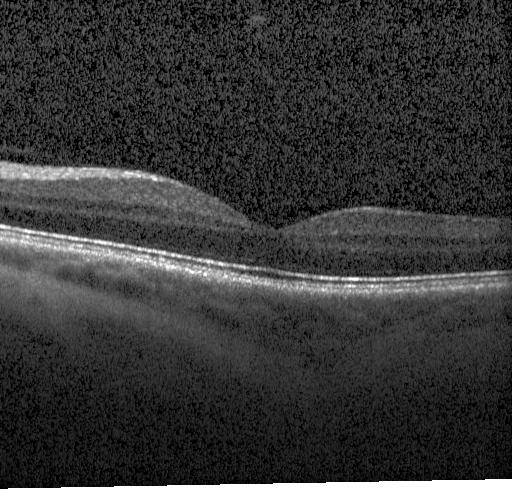

Spectral-domain OCT. Optical coherence tomography B-scan. Heidelberg Spectralis OCT system. Diagnosis: no CNV, DME, or drusen.